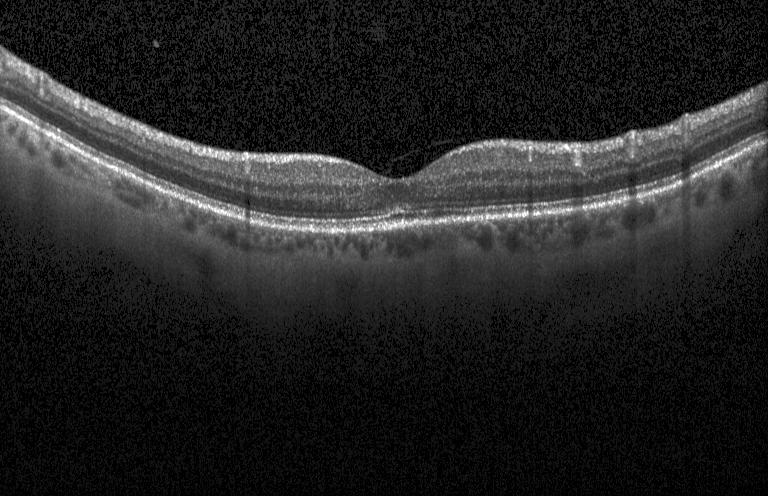

Retinal OCT cross-section — The scan shows neither choroidal neovascularization, diabetic macular edema, nor drusen.